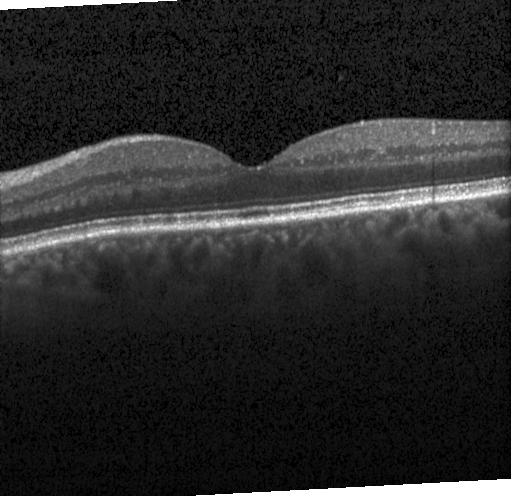

Heidelberg Spectralis; fovea-centered; SD-OCT; retinal OCT cross-section.
Macular OCT: neither choroidal neovascularization, diabetic macular edema, nor drusen.